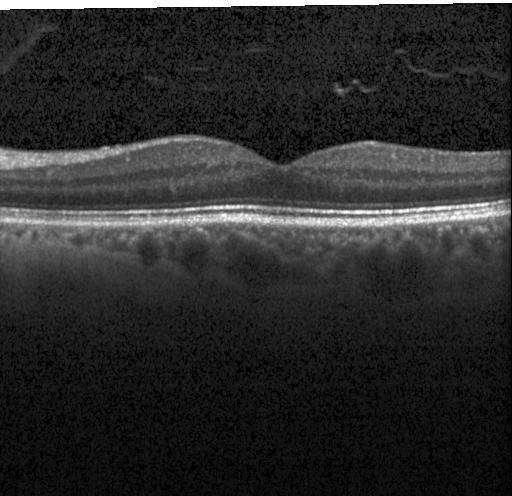

This B-scan demonstrates neither choroidal neovascularization, diabetic macular edema, nor drusen.